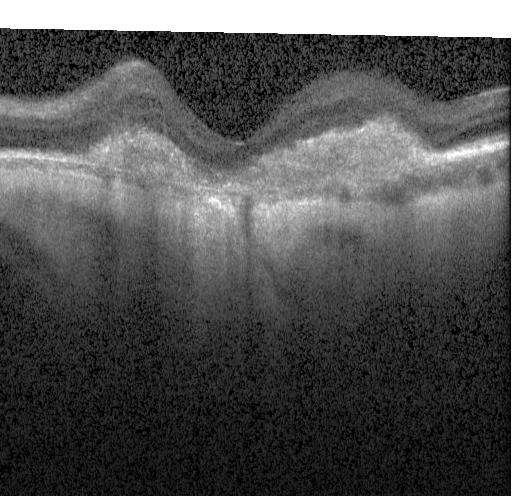

Retinal OCT B-scan · macular scan · spectral-domain OCT
Diagnosis: a choroidal neovascular membrane.